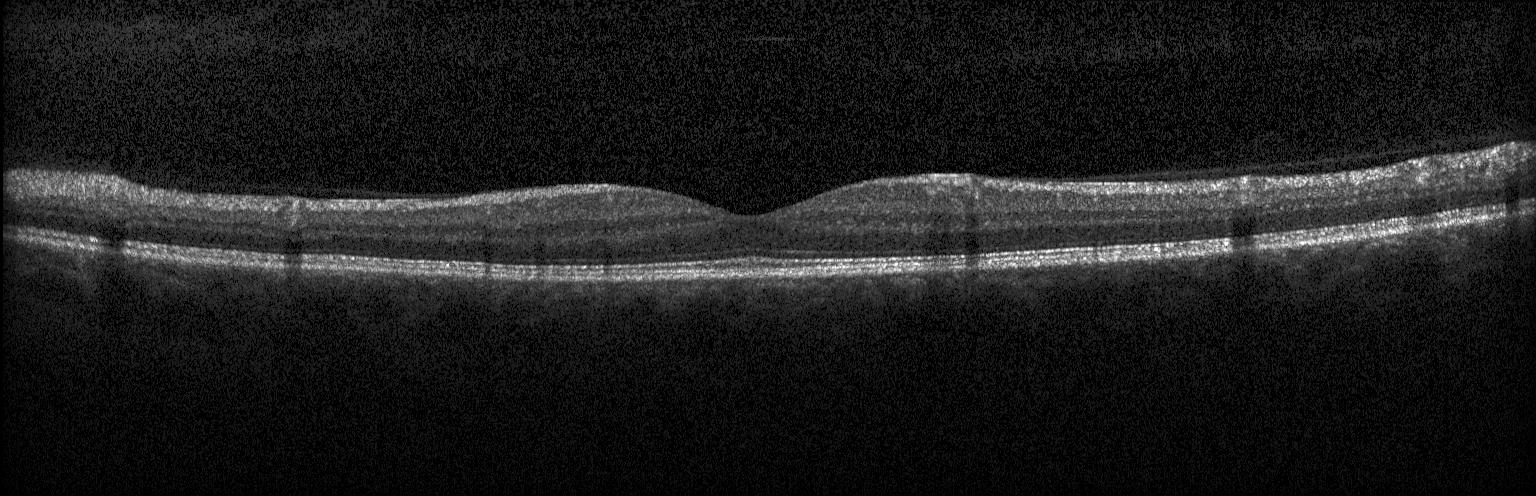

Optical coherence tomography scan. Macular scan — Diagnosis: no evidence of choroidal neovascularization, diabetic macular edema, or drusen.